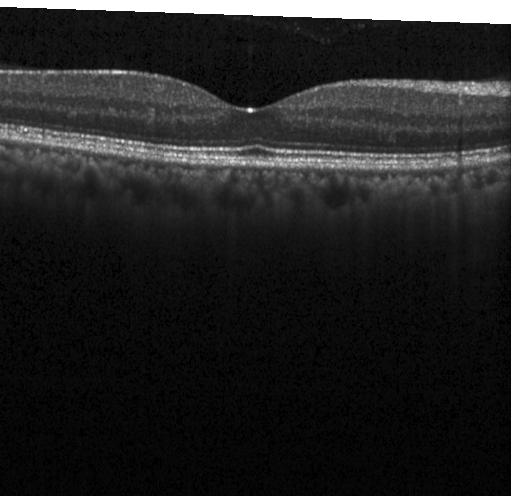 Diagnosis: no choroidal neovascularization, no diabetic macular edema, and no drusen.